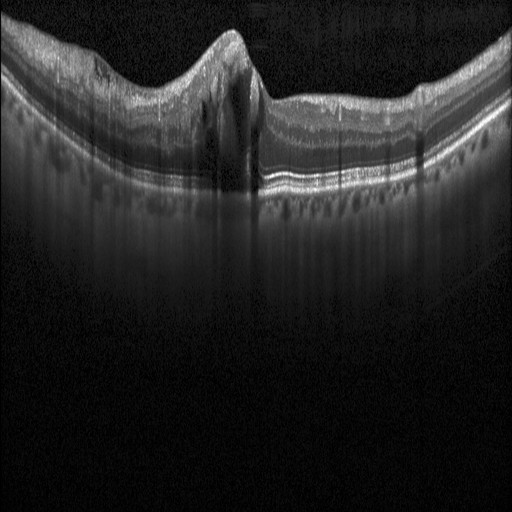
OCT line scan.
Finding: DME.